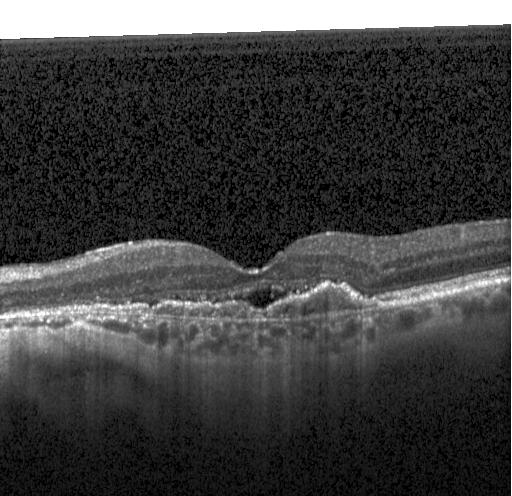

Retinal OCT cross-section
Finding: a choroidal neovascular membrane.